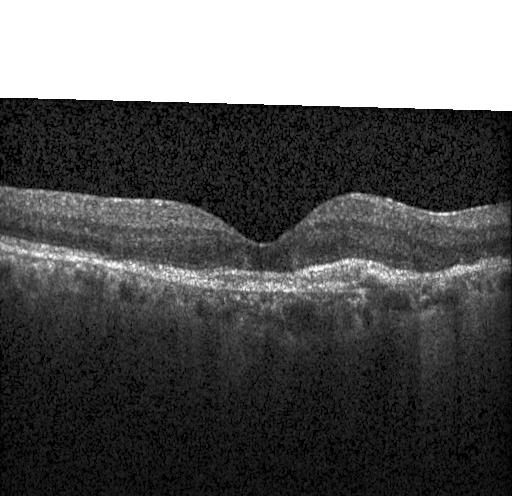
Diagnosis: choroidal neovascularization.